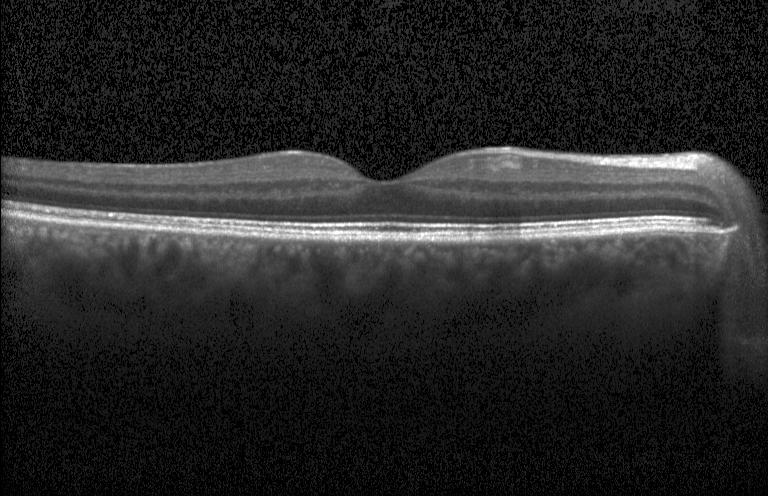 OCT finding: no CNV, DME, or drusen.